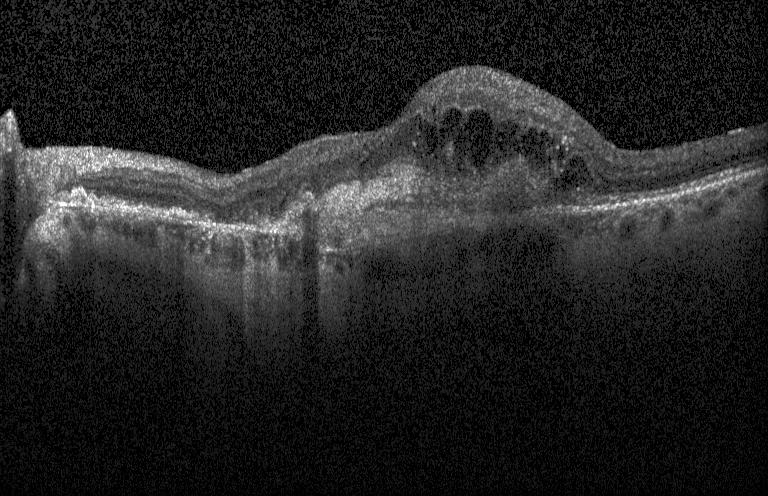
Retinal OCT B-scan. This B-scan demonstrates CNV.